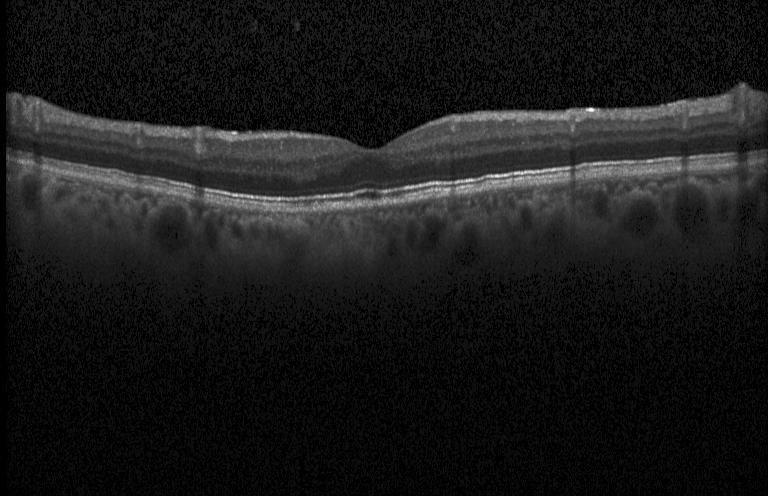 SD-OCT. Heidelberg Spectralis OCT system. Optical coherence tomography B-scan.
This B-scan demonstrates no choroidal neovascularization, diabetic macular edema, or drusen.